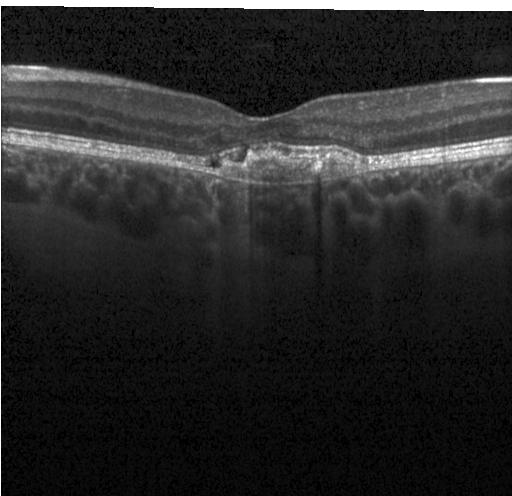
Retinal OCT B-scan; Heidelberg Spectralis OCT system — Assessment: choroidal neovascularization (CNV).